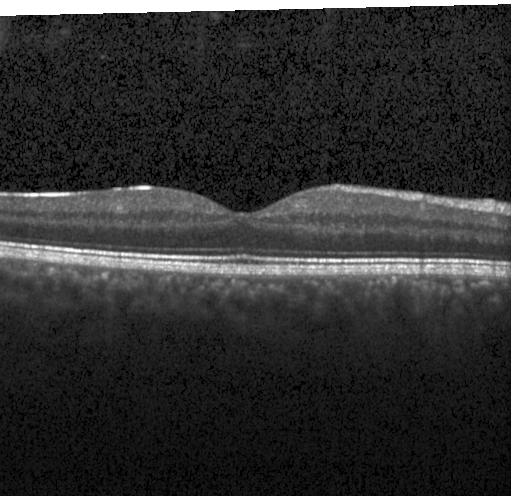 Macular OCT: neither choroidal neovascularization, diabetic macular edema, nor drusen.